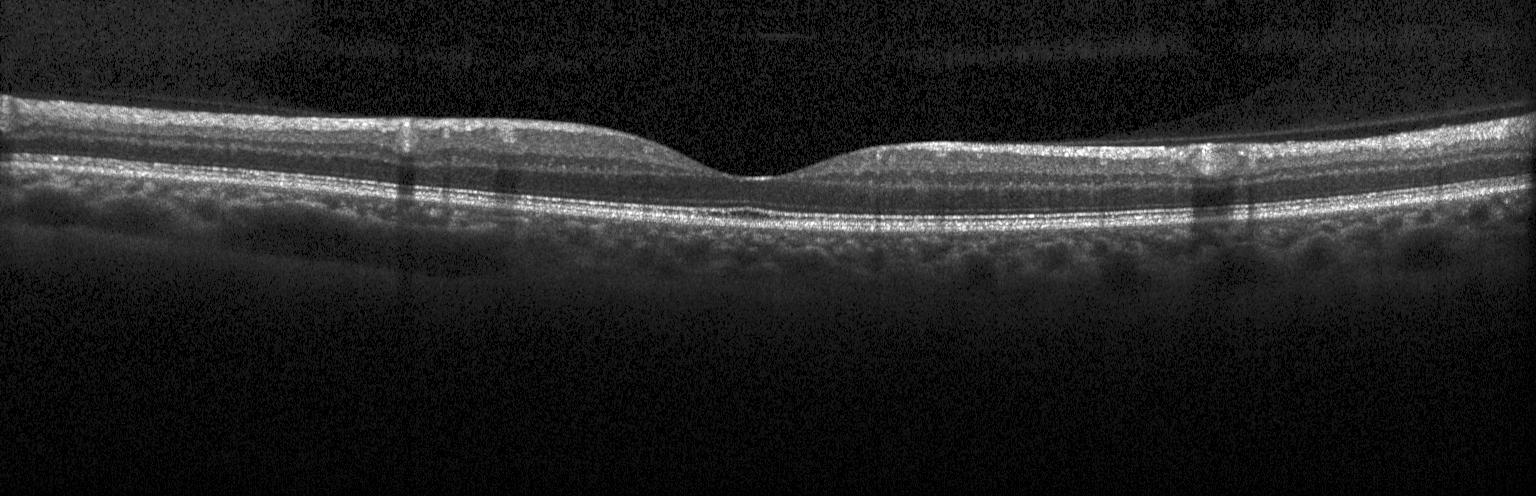
Diagnosis: neither CNV, DME, nor drusen.